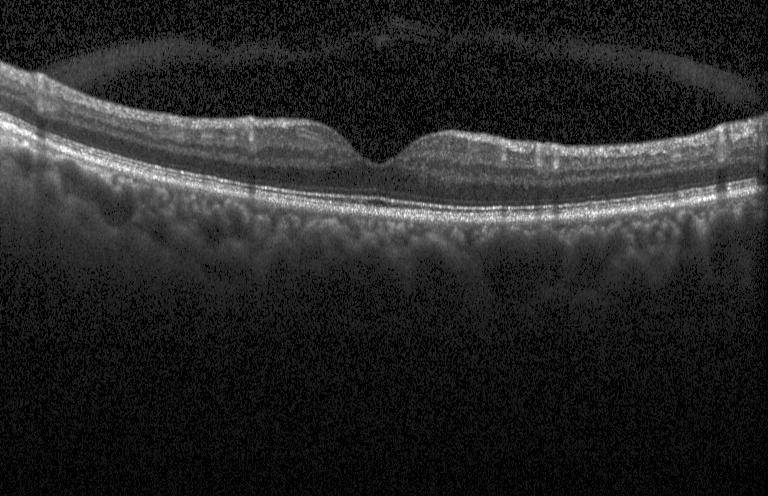 Retinal OCT cross-section showing neither choroidal neovascularization, diabetic macular edema, nor drusen.